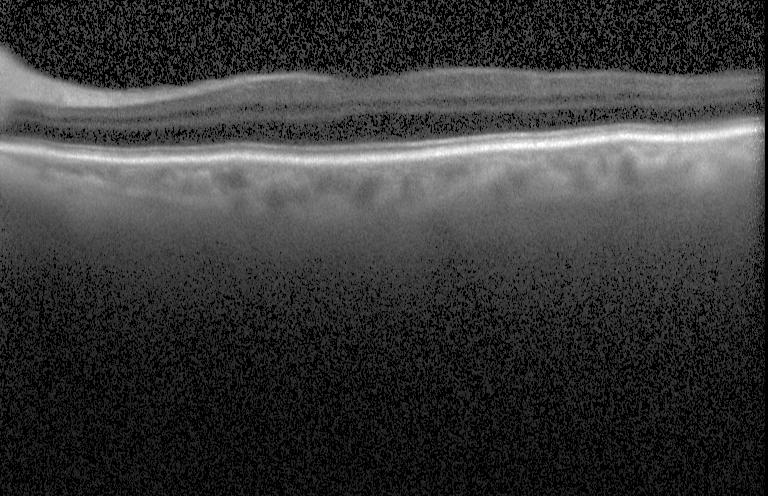

Optical coherence tomography B-scan
Assessment: no evidence of choroidal neovascularization, diabetic macular edema, or drusen.